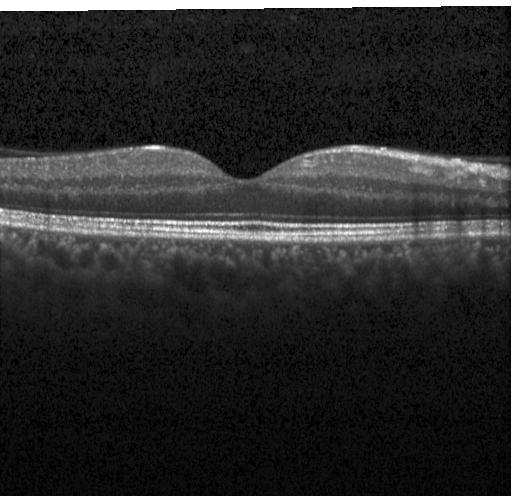
Spectral-domain optical coherence tomography · Heidelberg Spectralis OCT system · optical coherence tomography B-scan. Finding: no choroidal neovascularization, diabetic macular edema, or drusen.